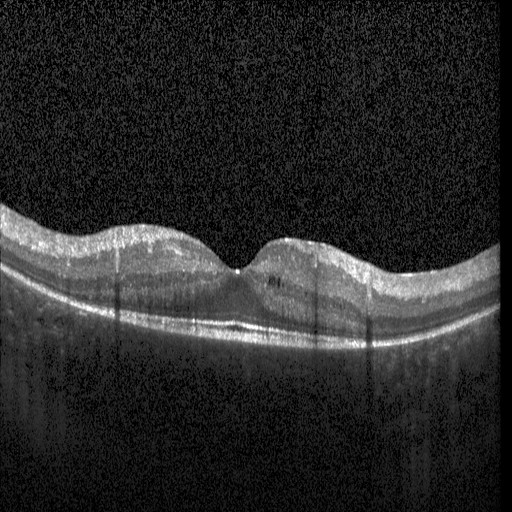 Retinal OCT B-scan
Impression: diabetic macular edema (DME).